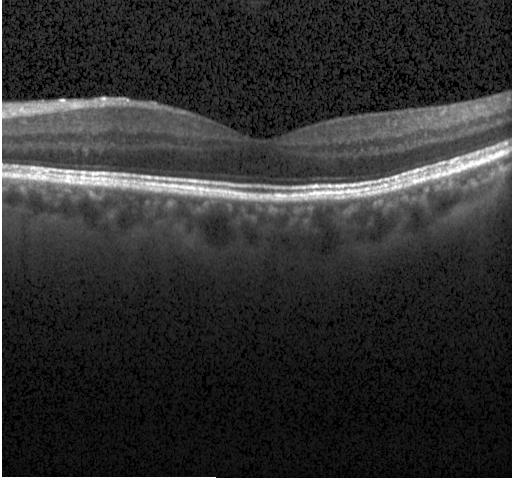

OCT B-scan showing no CNV, no DME, and no drusen.